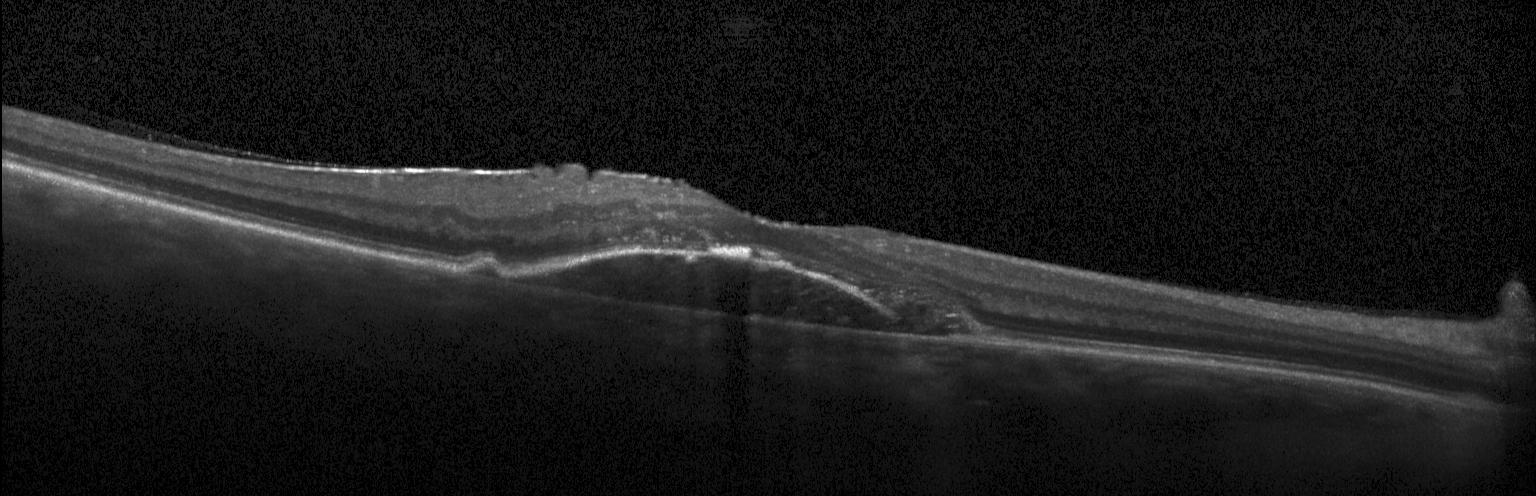 Centered on the fovea; optical coherence tomography scan.
Assessment: a choroidal neovascular membrane.